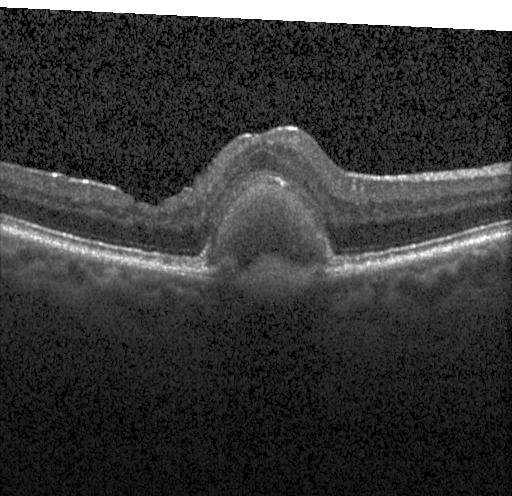 Macular OCT: a choroidal neovascular membrane.